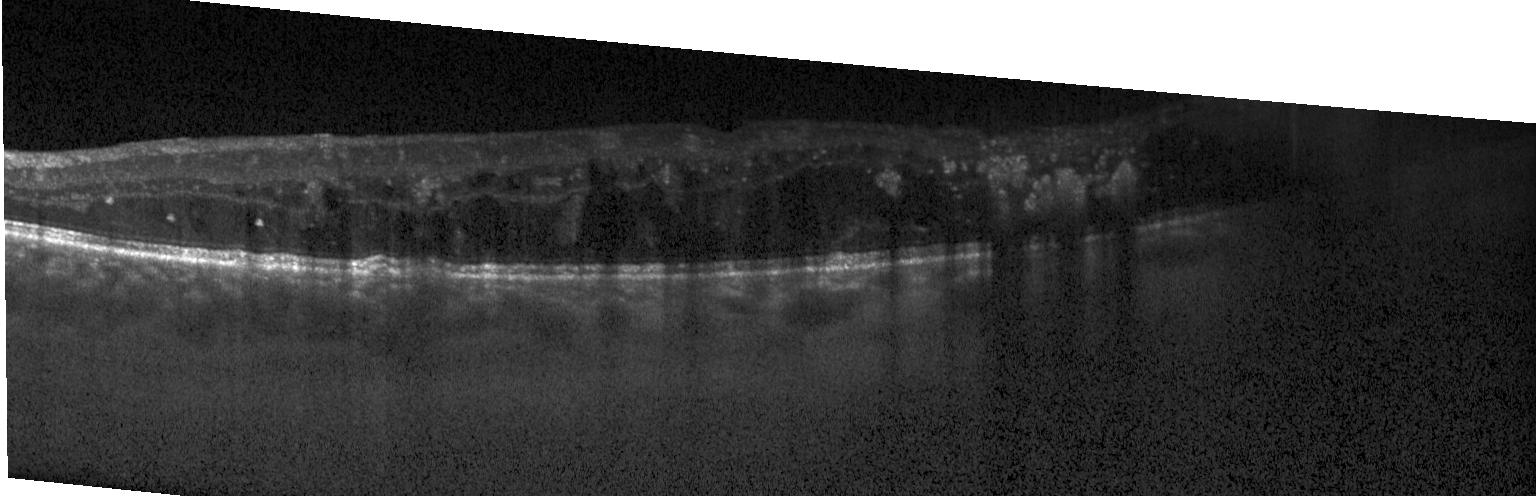

OCT B-scan. Finding: DME.